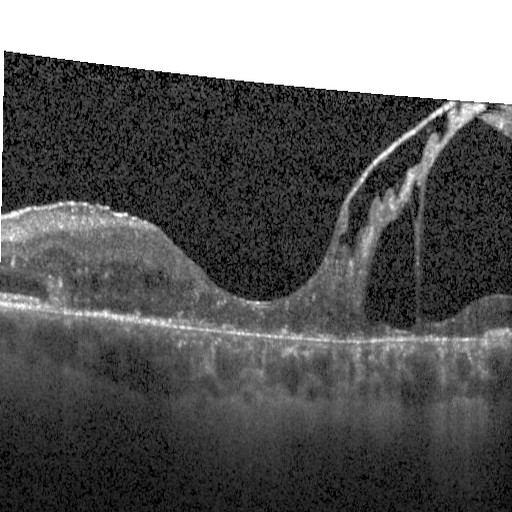
OCT scan showing diabetic macular edema.